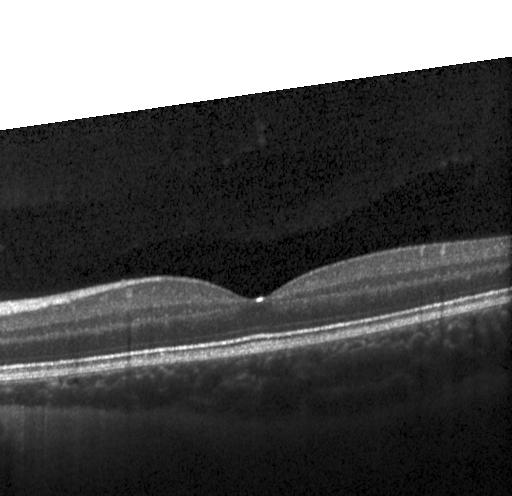 Macular OCT: neither choroidal neovascularization, diabetic macular edema, nor drusen.